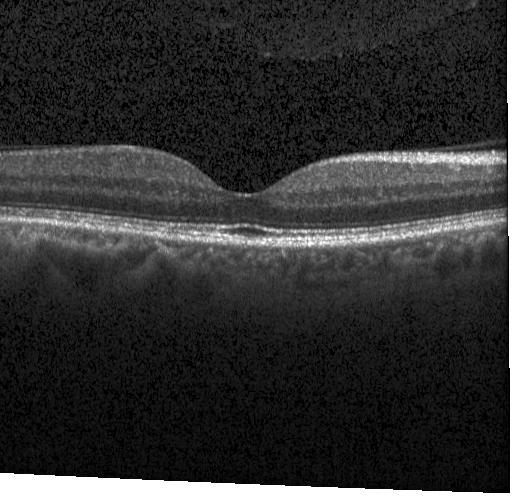

Through the macula, retinal OCT cross-section, SD-OCT. Assessment: no evidence of CNV, DME, or drusen.